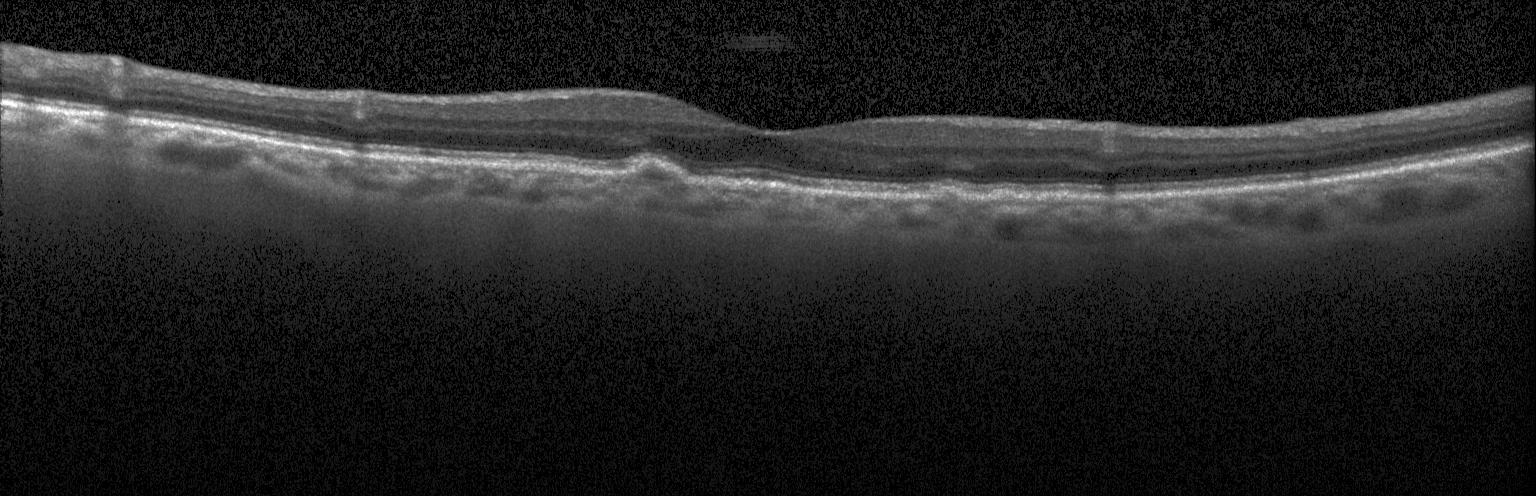
Retinal OCT cross-section showing sub-RPE drusenoid deposits.